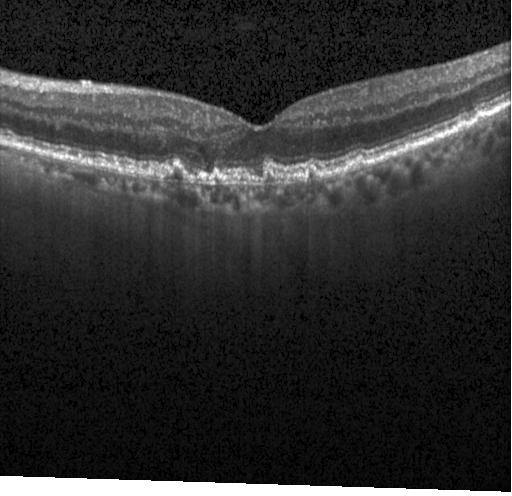

OCT line scan. Through the macula. Instrument: Heidelberg Spectralis. Spectral-domain OCT
Macular OCT: sub-RPE drusenoid deposits.